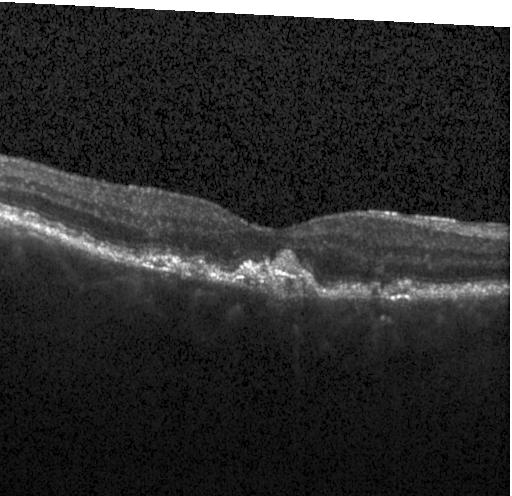

Retinal OCT B-scan. Instrument: Heidelberg Spectralis. Centered on the fovea. SD-OCT.
Choroidal neovascularization.